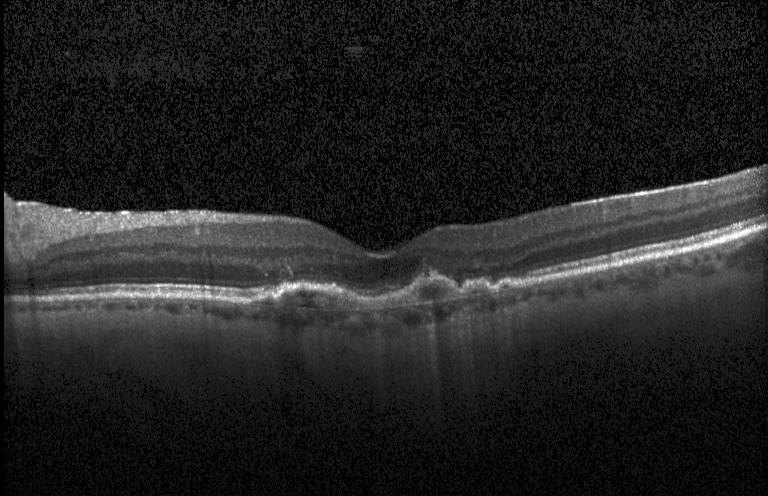 OCT B-scan. Spectral-domain optical coherence tomography. Macular scan.
Diagnosis: a choroidal neovascular membrane.